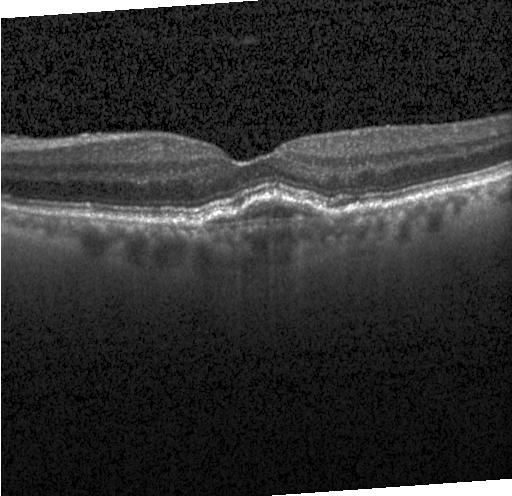
Spectral-domain OCT; retinal OCT cross-section; centered on the fovea; Heidelberg Spectralis.
A choroidal neovascular membrane.